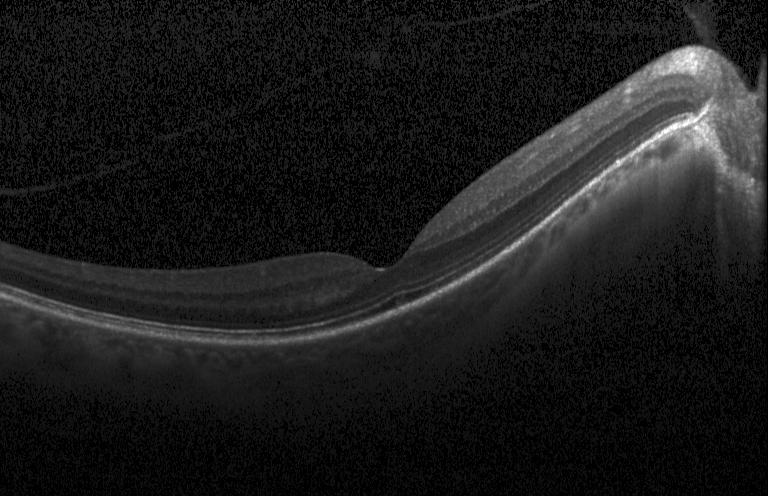

Dx: no choroidal neovascularization, diabetic macular edema, or drusen.